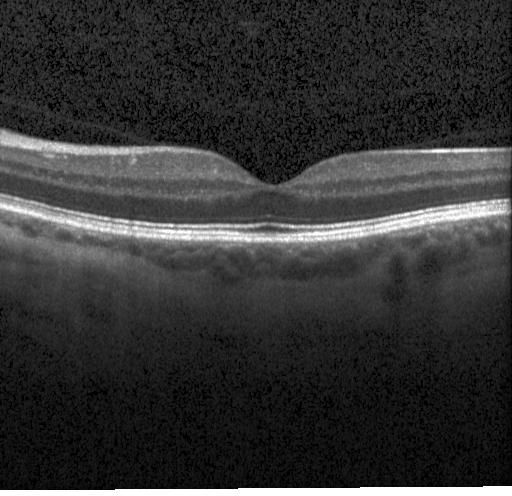
Acquired on a Heidelberg Spectralis, retinal OCT cross-section.
Impression: neither choroidal neovascularization, diabetic macular edema, nor drusen.